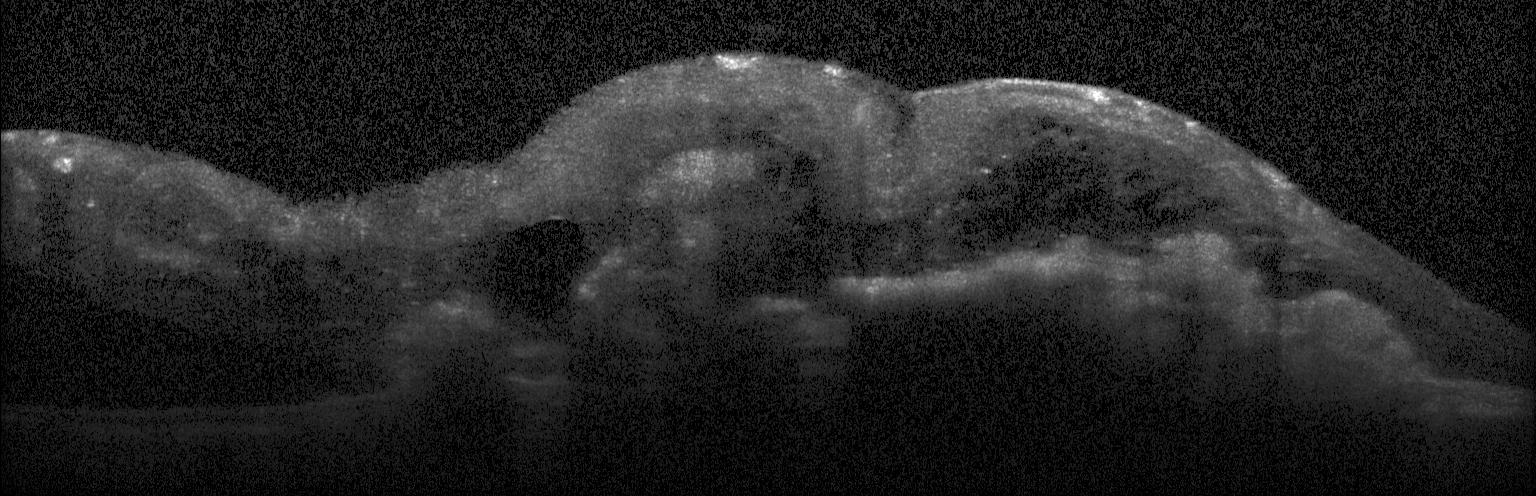 OCT finding: CNV.